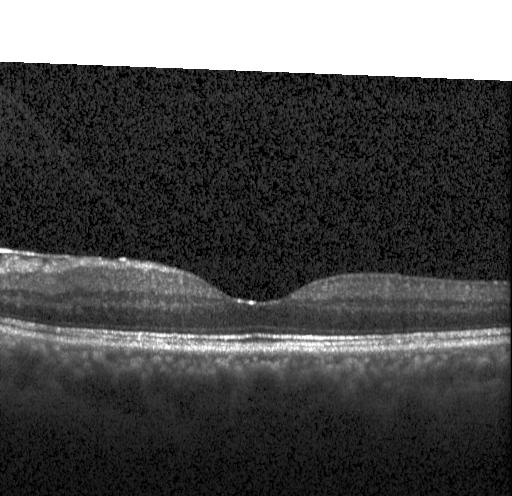

SD-OCT; retinal OCT B-scan; through the macula; instrument: Heidelberg Spectralis
Diagnosis: no choroidal neovascularization, no diabetic macular edema, and no drusen.